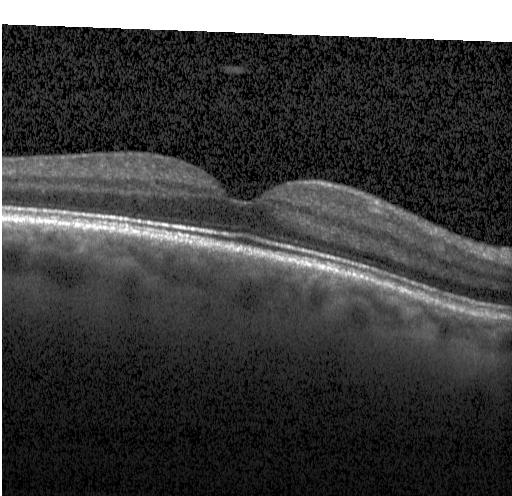

Heidelberg Spectralis, retinal OCT B-scan — Finding: no choroidal neovascularization, diabetic macular edema, or drusen.